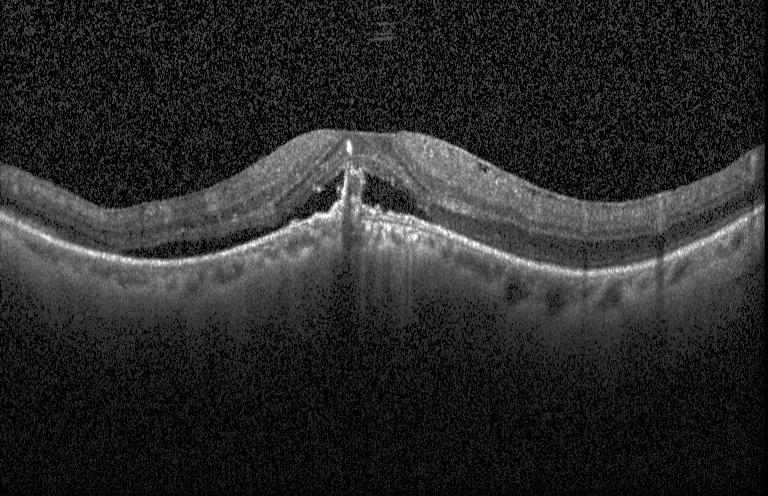
Through the macula. Retinal OCT B-scan — Impression: choroidal neovascularization.